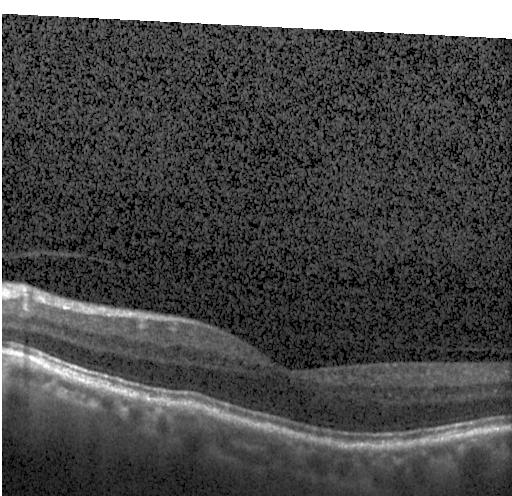

No evidence of CNV, DME, or drusen.